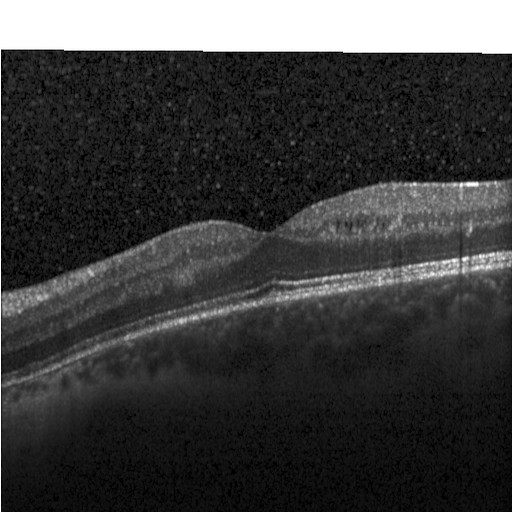 OCT line scan; macular scan; spectral-domain OCT.
Dx: DME.